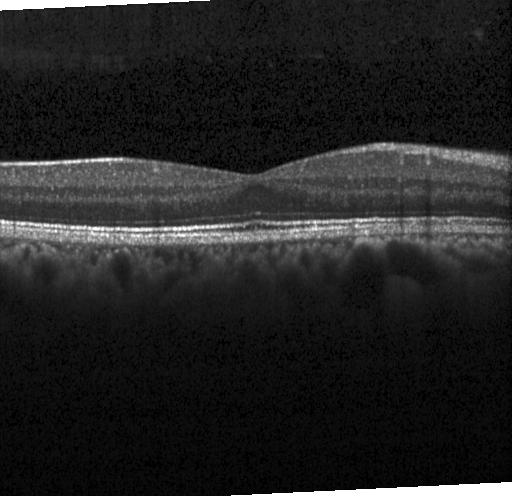
Retinal OCT cross-section.
Finding: no choroidal neovascularization, diabetic macular edema, or drusen.